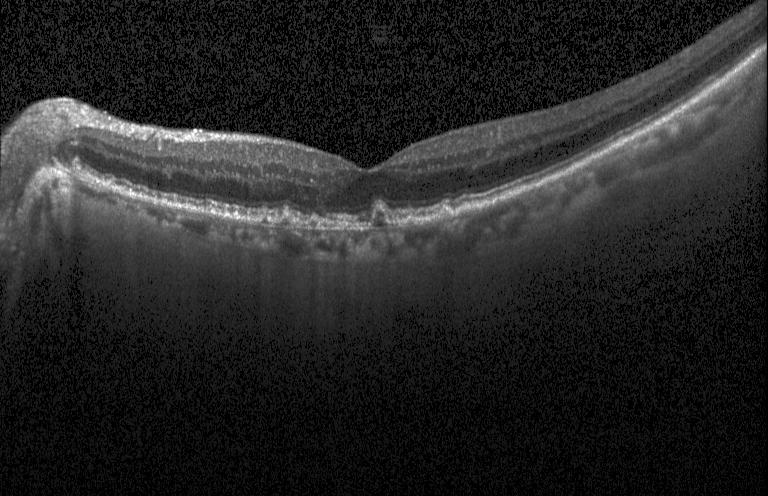 Macular scan; instrument: Heidelberg Spectralis; OCT B-scan
OCT finding: a choroidal neovascular membrane.